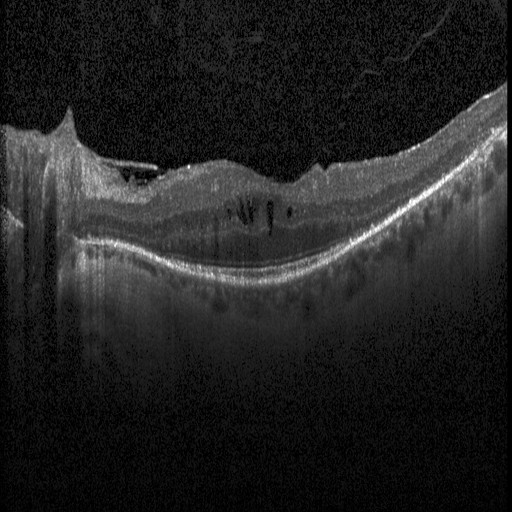 Horizontal scan through the fovea · retinal OCT B-scan · instrument: Heidelberg Spectralis.
Finding: DME.